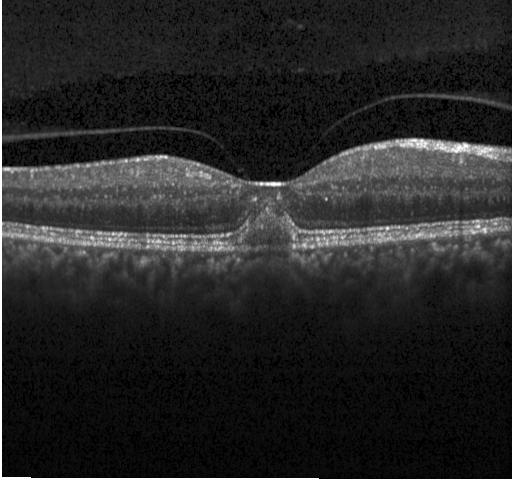

Diagnosis: CNV.